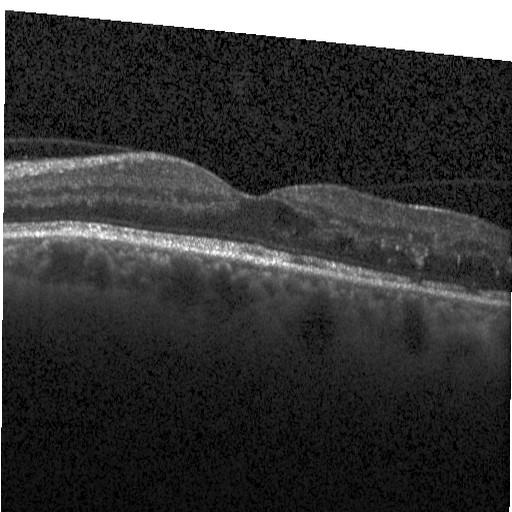

Acquired on a Heidelberg Spectralis. OCT line scan. Finding: diabetic macular edema (DME).